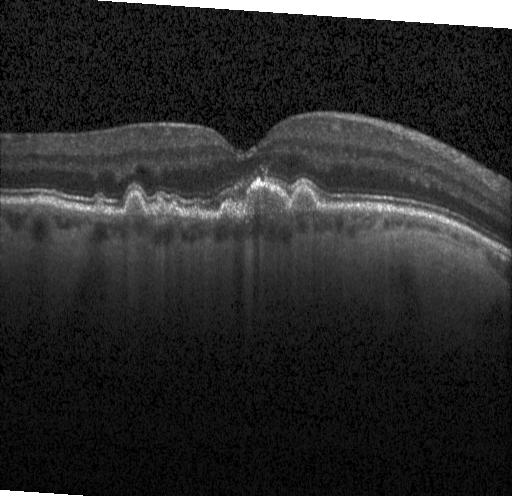

OCT line scan — Finding: sub-RPE drusenoid deposits.